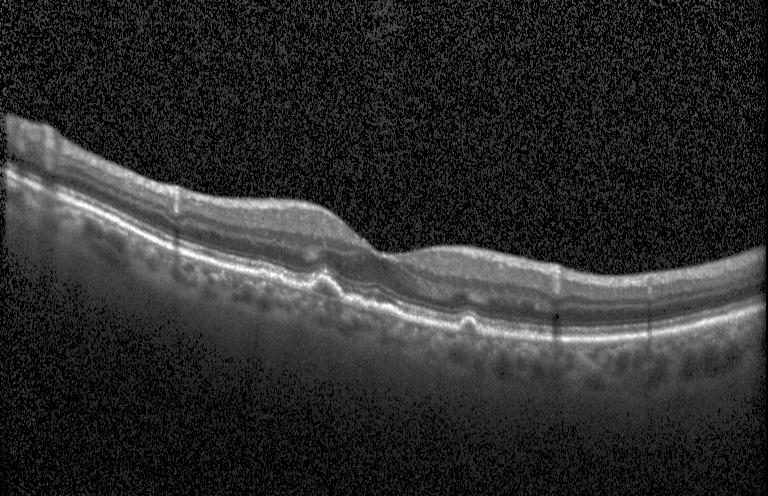 Macular OCT: drusen.